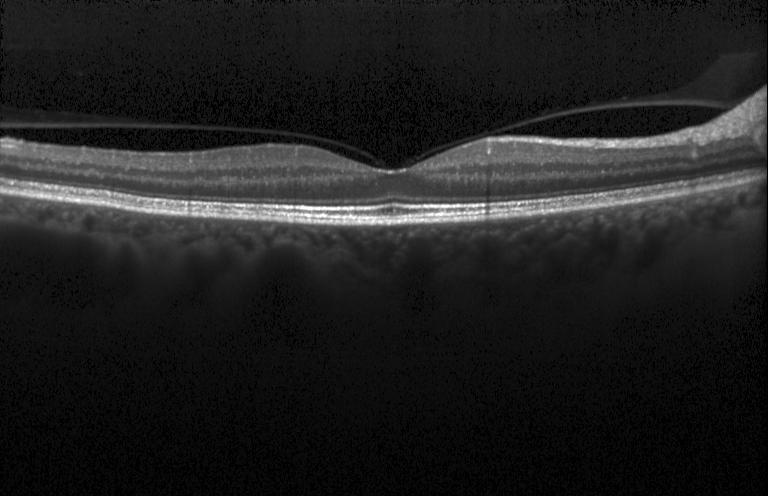
Finding: neither choroidal neovascularization, diabetic macular edema, nor drusen.